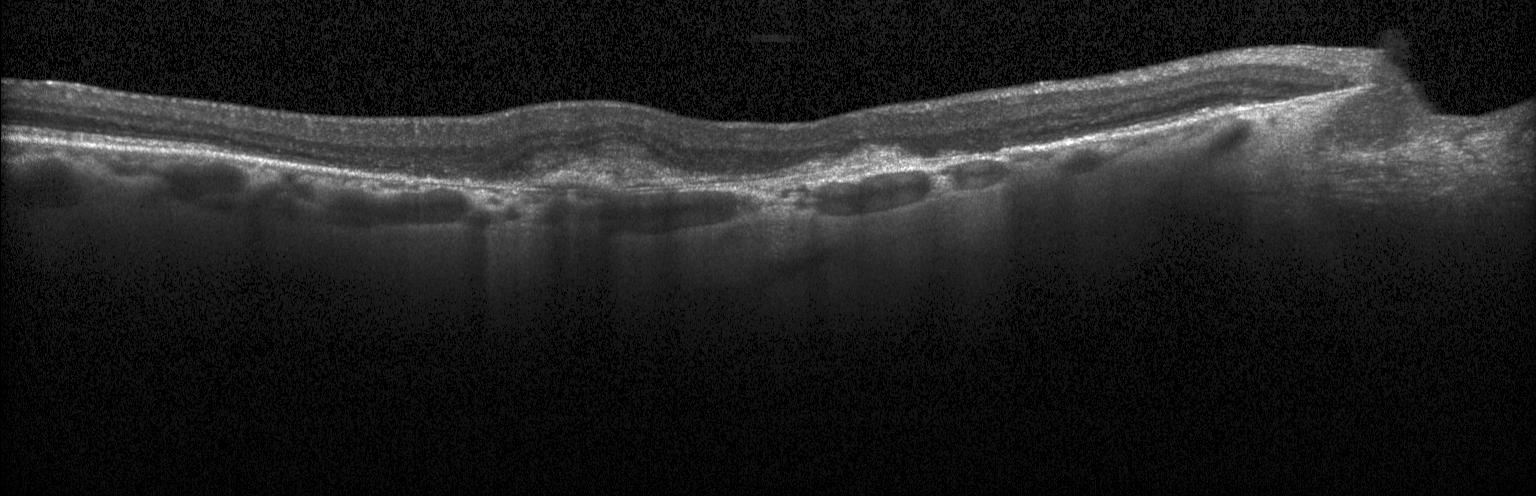

Instrument: Heidelberg Spectralis. Spectral-domain OCT. Centered on the fovea. Optical coherence tomography scan.
The scan shows a choroidal neovascular membrane.